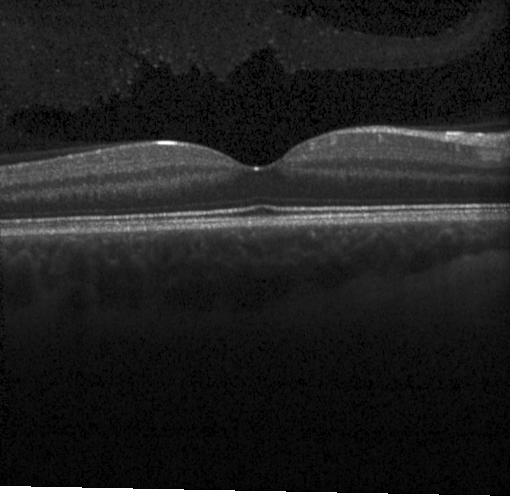

Optical coherence tomography scan, macular scan — No evidence of choroidal neovascularization, diabetic macular edema, or drusen.